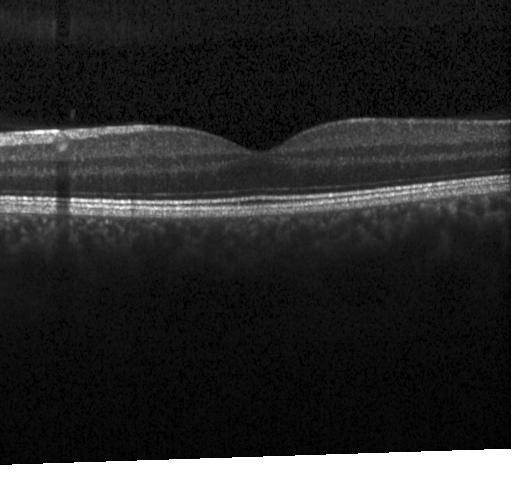
Heidelberg Spectralis; OCT B-scan. No CNV, DME, or drusen.